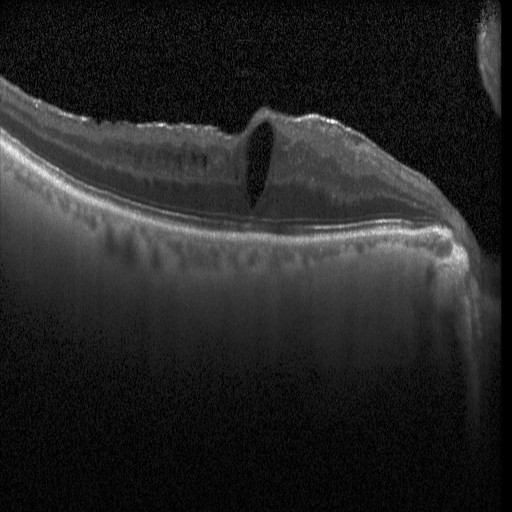
OCT B-scan. Assessment: diabetic macular edema.